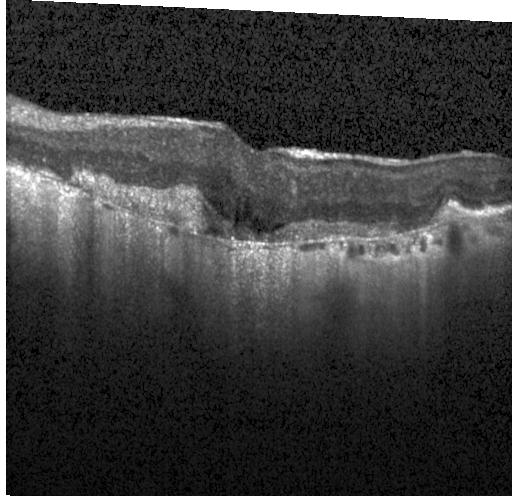
Heidelberg Spectralis. Centered on the fovea. OCT B-scan. SD-OCT.
Finding: a choroidal neovascular membrane.